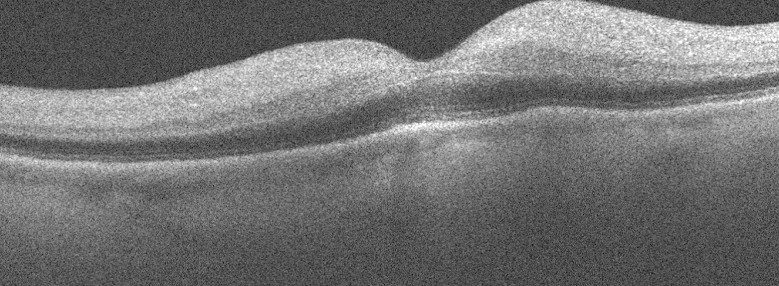
OCT line scan. Optovue Avanti RTVue XR. The scan shows retinal artery occlusion.